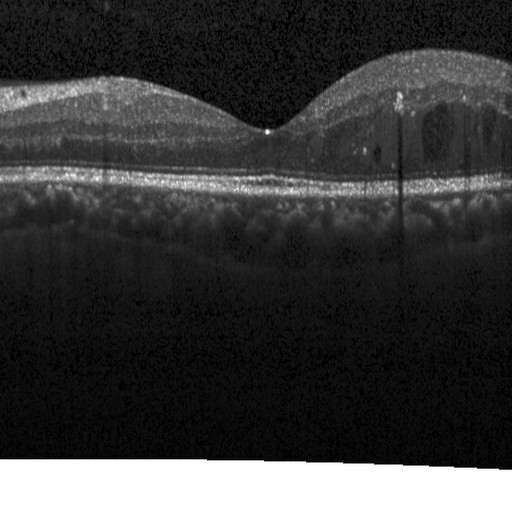

Centered on the fovea; acquired on a Heidelberg Spectralis; retinal OCT B-scan — Diabetic macular edema.